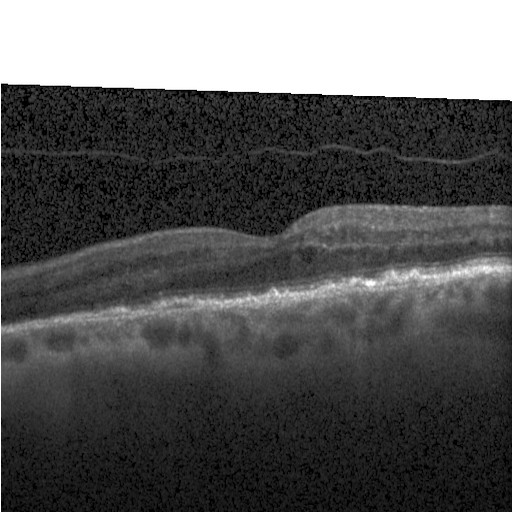 Assessment: diabetic macular edema.